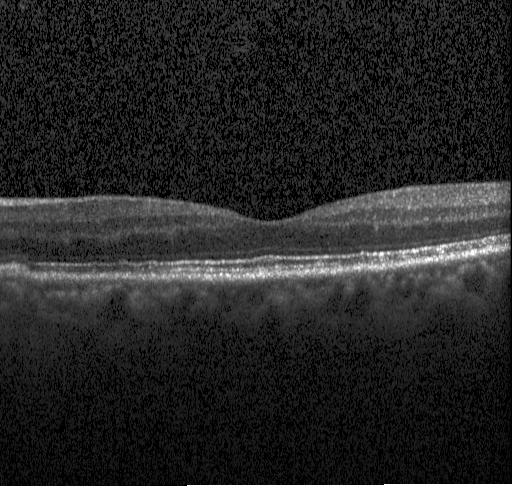
Diagnosis: drusen.